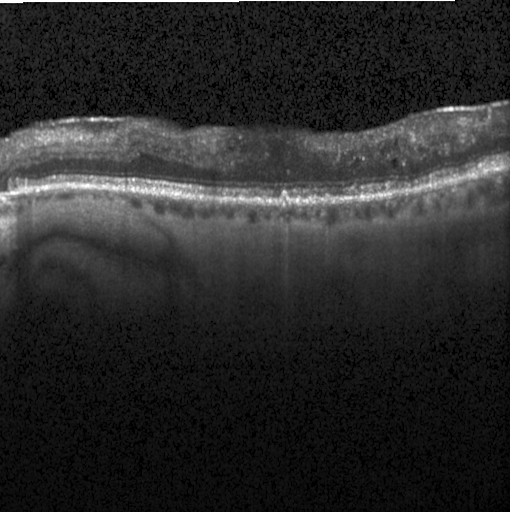

SD-OCT, OCT line scan. Diagnosis: diabetic macular edema.